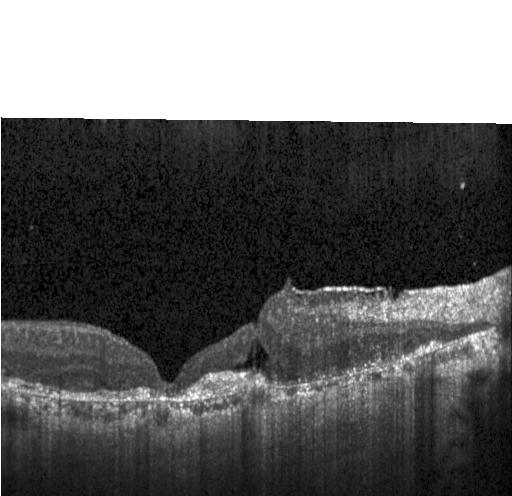 Finding: a choroidal neovascular membrane.